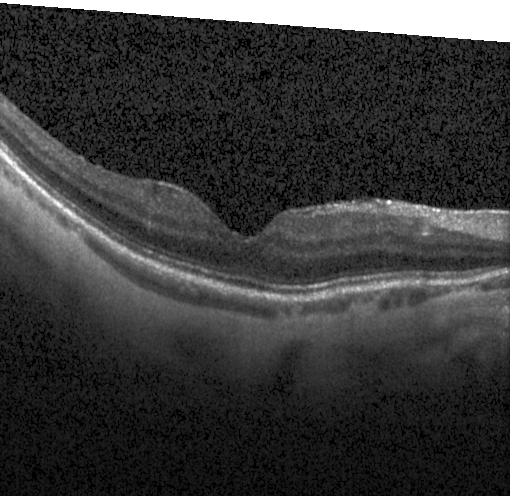 Spectral-domain OCT B-scan: no choroidal neovascularization, diabetic macular edema, or drusen.